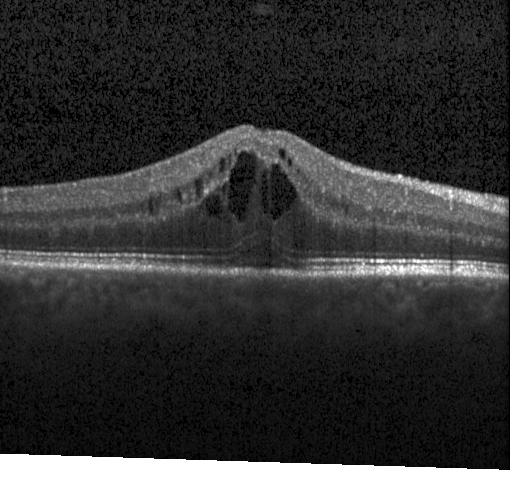 Retinal OCT B-scan · acquired on a Heidelberg Spectralis · spectral-domain optical coherence tomography · centered on the fovea.
Finding: diabetic macular edema (DME).